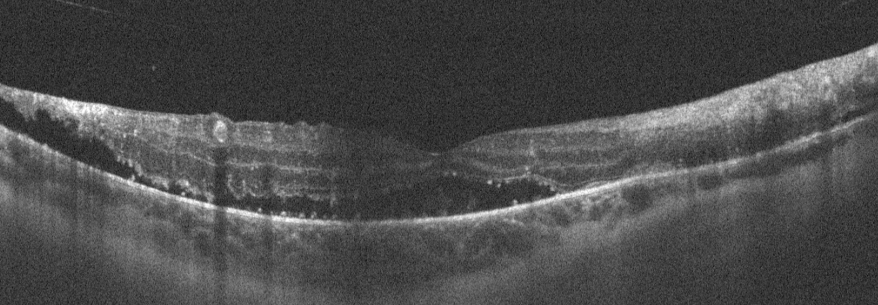
Retinal OCT cross-section — Finding: age-related macular degeneration.